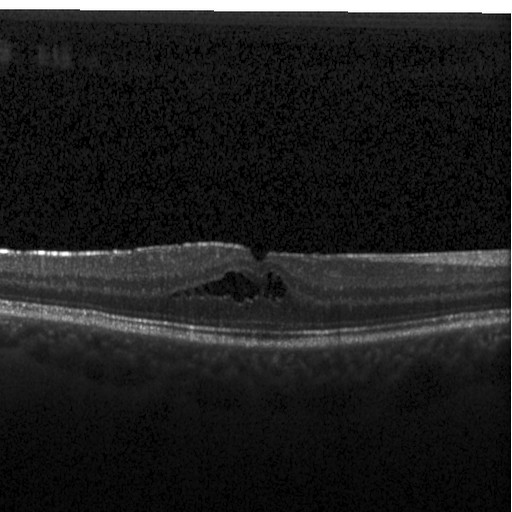 SD-OCT, centered on the fovea, Heidelberg Spectralis, OCT B-scan
Finding: DME.